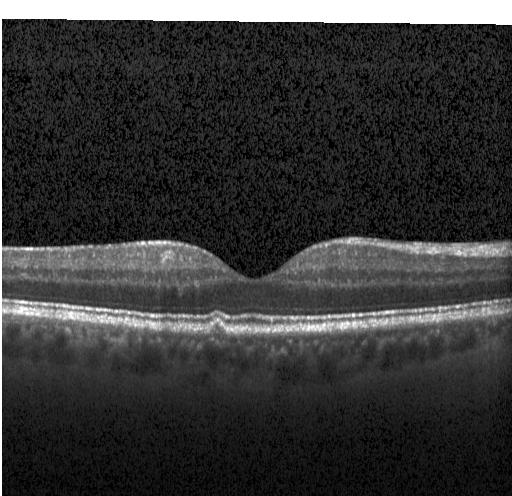
Retinal OCT cross-section.
Sub-RPE drusenoid deposits.